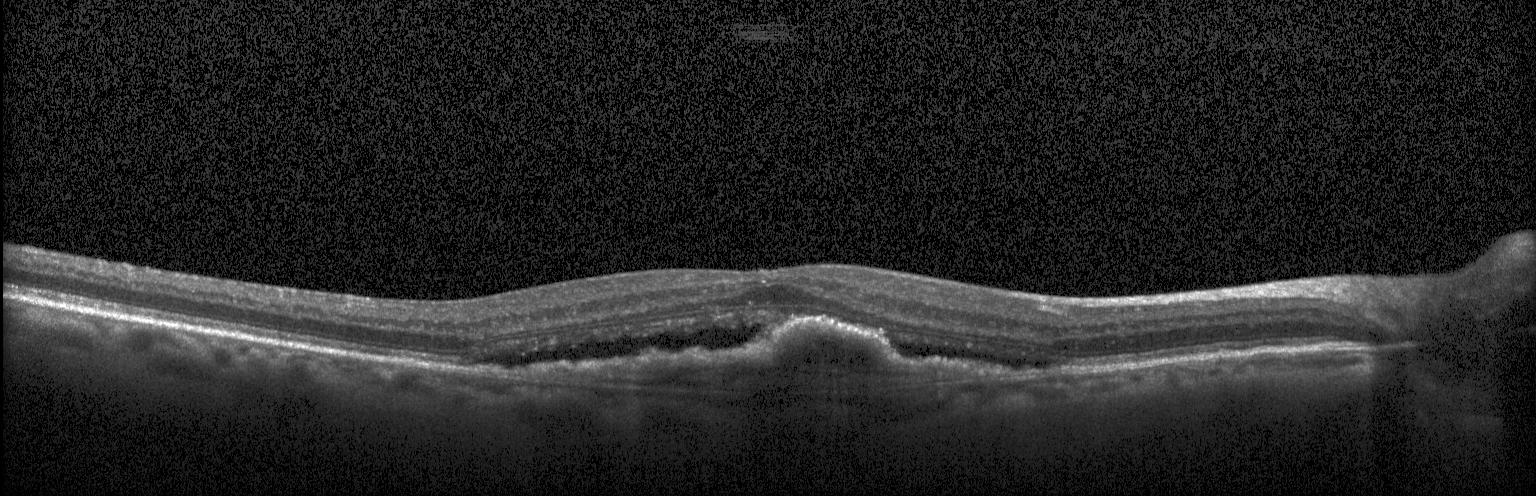 Retinal OCT cross-section · spectral-domain OCT
Finding: choroidal neovascularization (CNV).